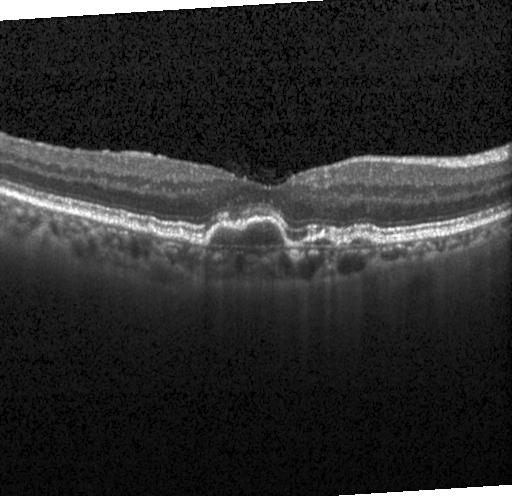
Dx: a choroidal neovascular membrane.